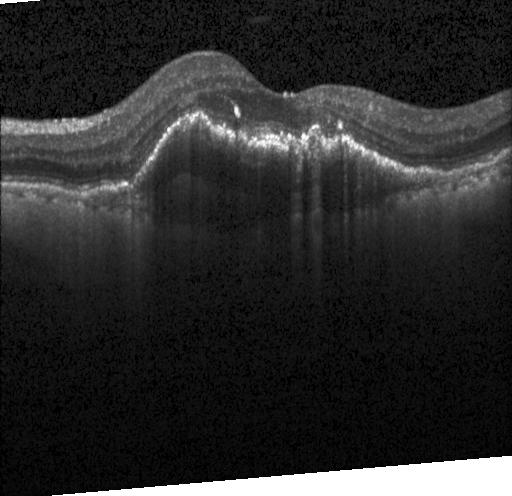 OCT B-scan showing CNV.